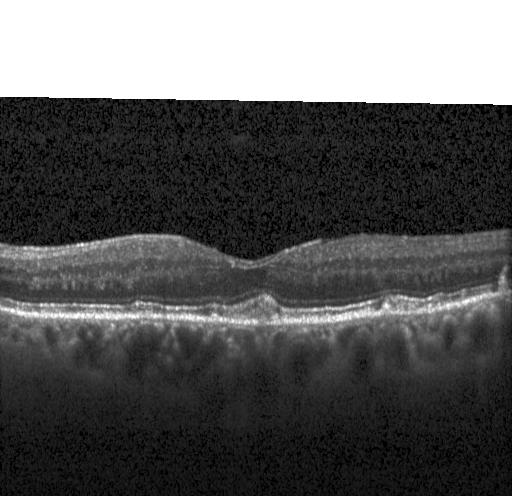

Optical coherence tomography B-scan
Diagnosis: drusen.